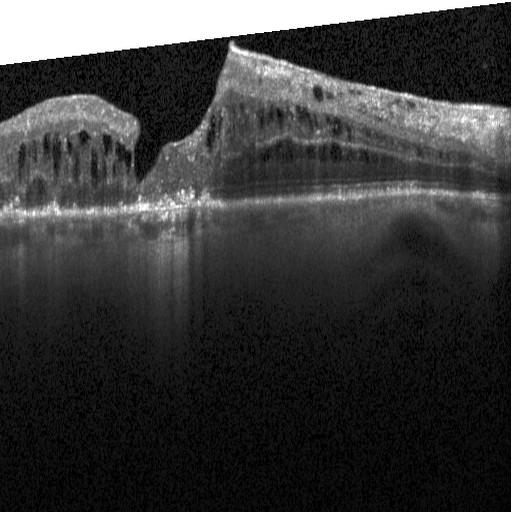
Retinal OCT B-scan — This B-scan demonstrates diabetic macular edema.